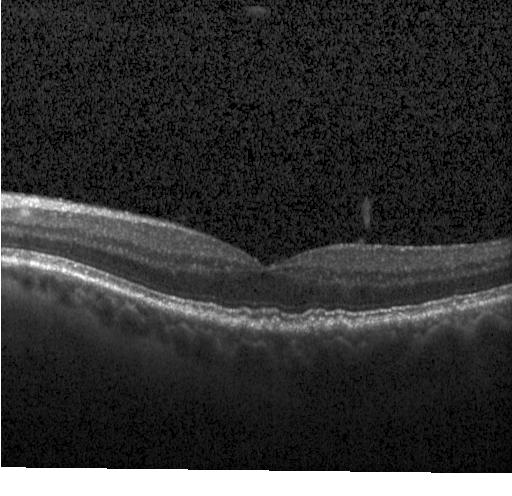
Retinal OCT B-scan; spectral-domain optical coherence tomography; Heidelberg Spectralis; horizontal scan through the fovea. Macular OCT: multiple drusen.